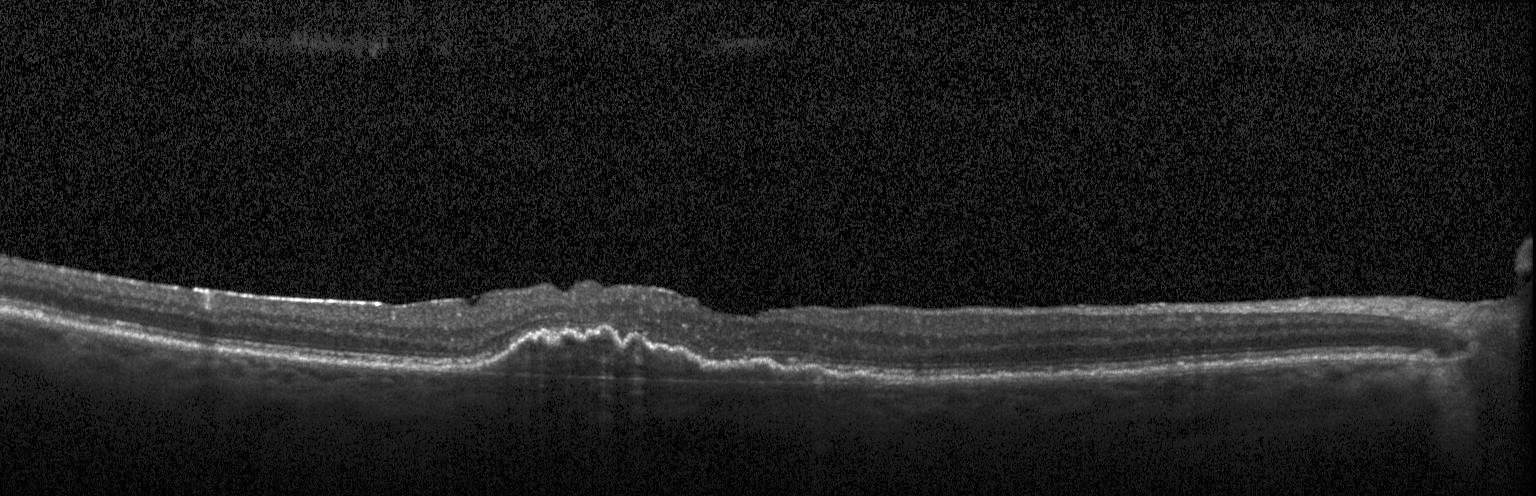 Heidelberg Spectralis OCT system, OCT line scan. The scan shows a choroidal neovascular membrane.